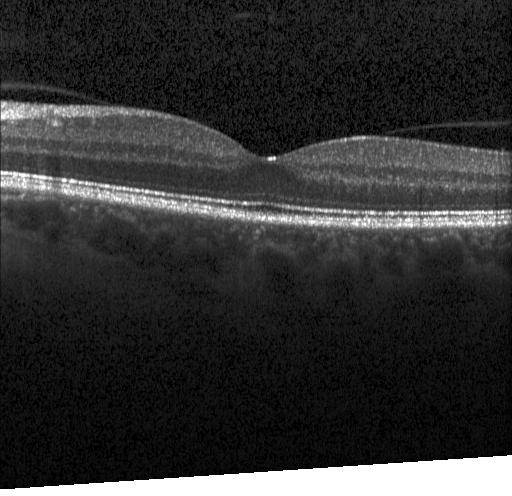
Finding: no evidence of choroidal neovascularization, diabetic macular edema, or drusen.